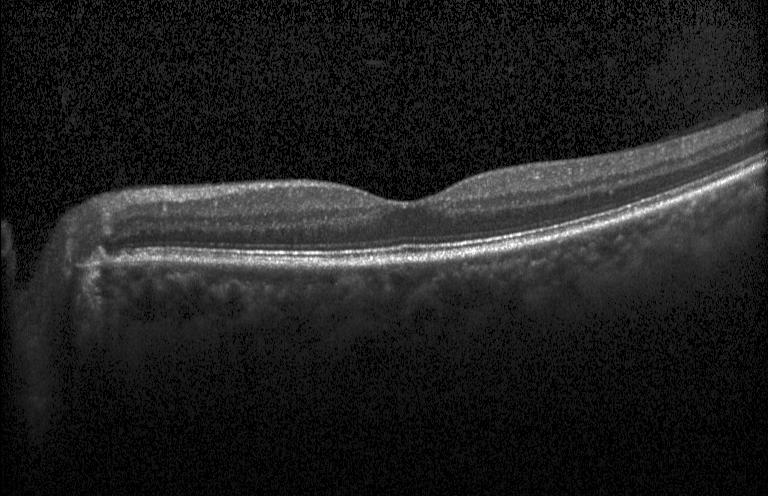

No CNV, DME, or drusen.